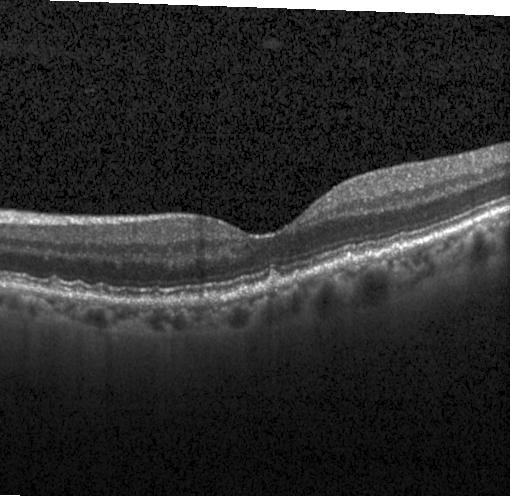 Dx: multiple drusen.